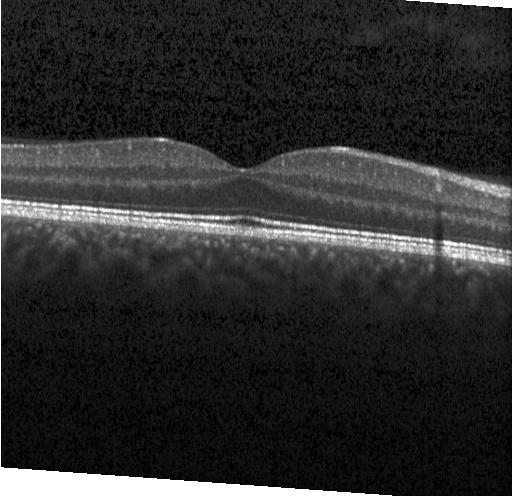

OCT B-scan showing no choroidal neovascularization, diabetic macular edema, or drusen.